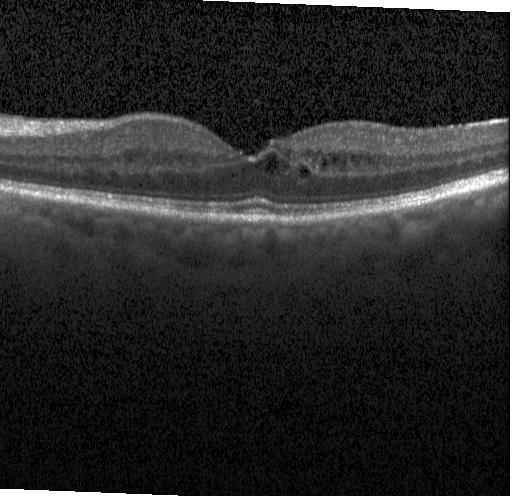

Through the macula, optical coherence tomography scan.
OCT finding: diabetic macular edema.